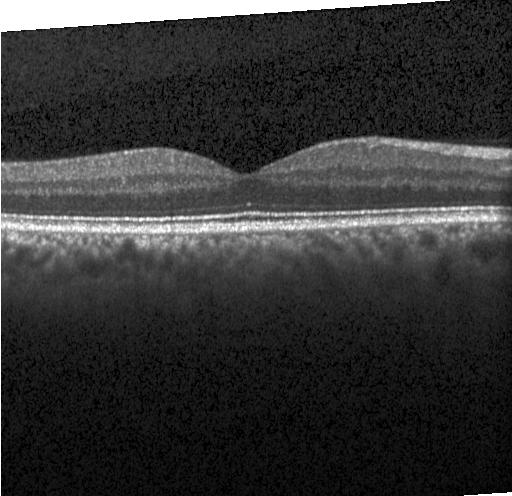
Optical coherence tomography scan. This B-scan demonstrates no evidence of CNV, DME, or drusen.